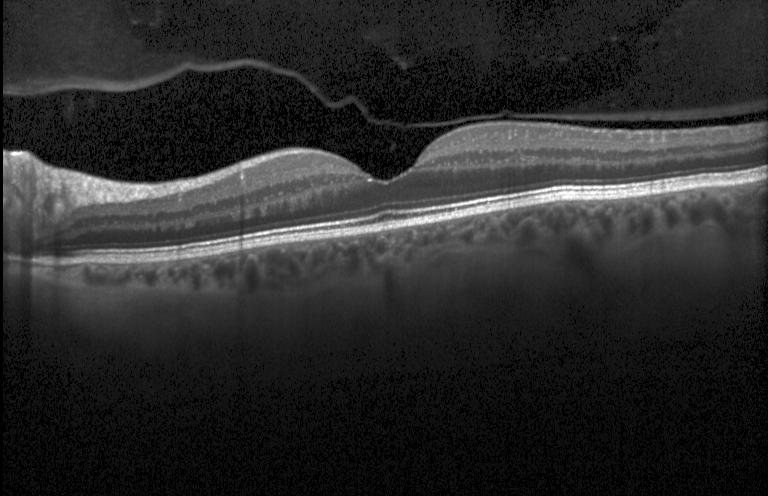
No evidence of CNV, DME, or drusen.